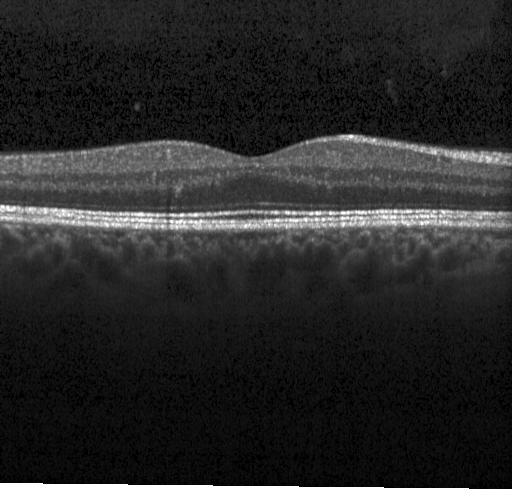 Macular scan; OCT B-scan.
Dx: no evidence of choroidal neovascularization, diabetic macular edema, or drusen.